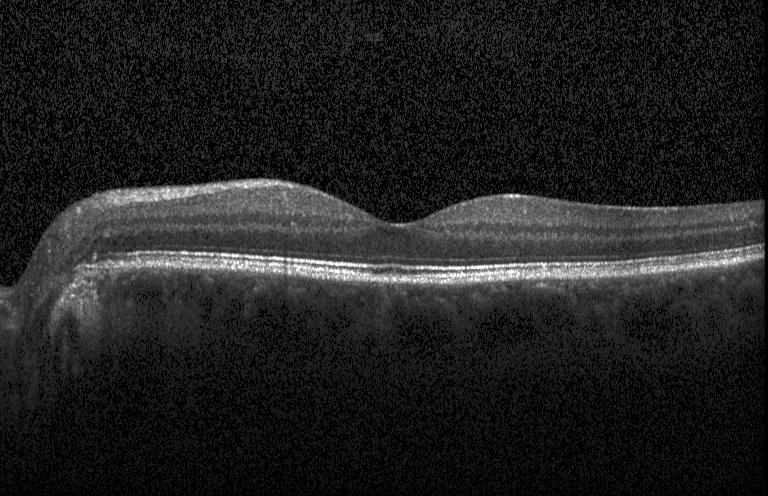
Spectral-domain OCT · OCT B-scan. Diagnosis: neither choroidal neovascularization, diabetic macular edema, nor drusen.